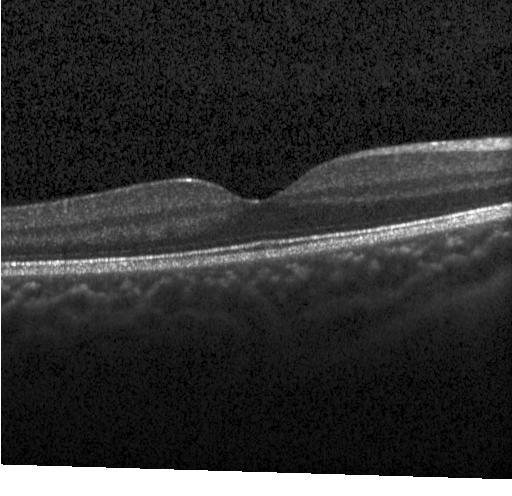 OCT B-scan; acquired on a Heidelberg Spectralis.
The scan shows no choroidal neovascularization, diabetic macular edema, or drusen.